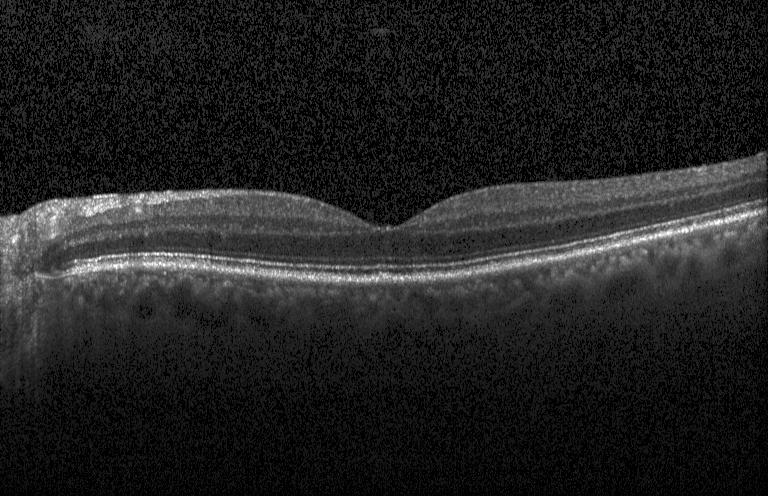 Spectral-domain optical coherence tomography, OCT line scan, horizontal scan through the fovea. Diagnosis: no choroidal neovascularization, diabetic macular edema, or drusen.